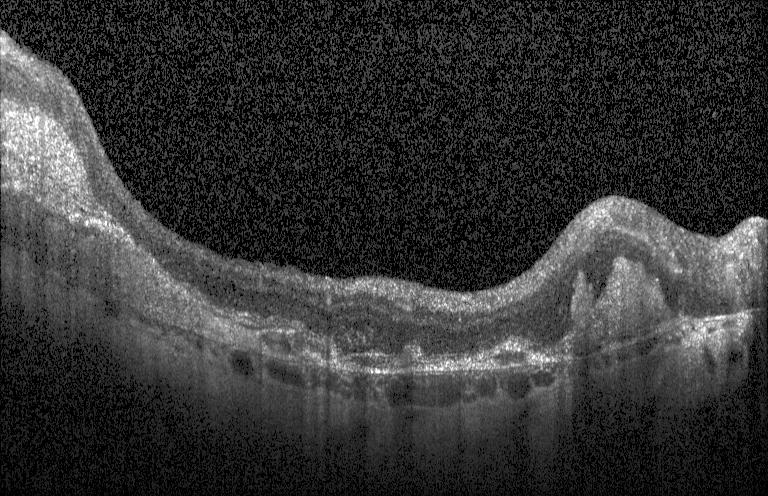 Finding: a choroidal neovascular membrane.